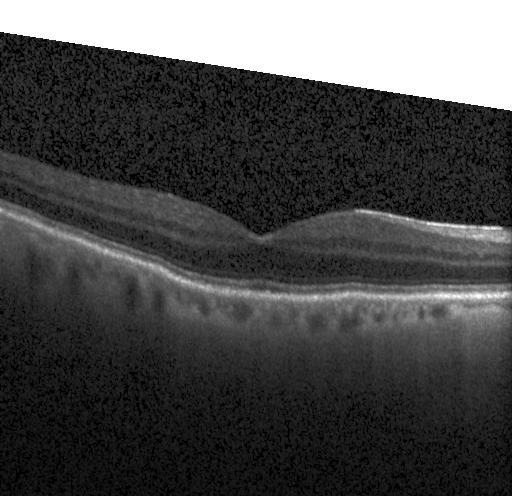 No choroidal neovascularization, no diabetic macular edema, and no drusen.